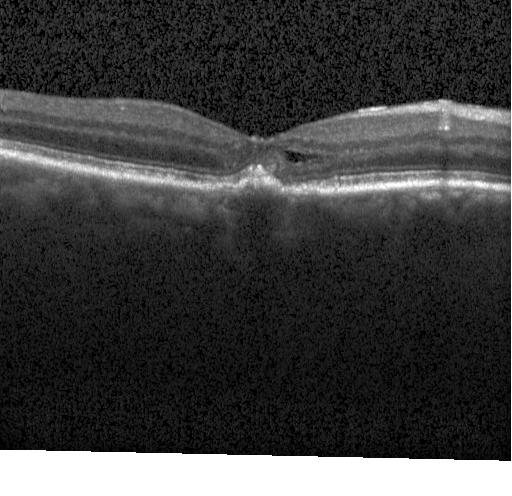 Retinal OCT cross-section showing a choroidal neovascular membrane.